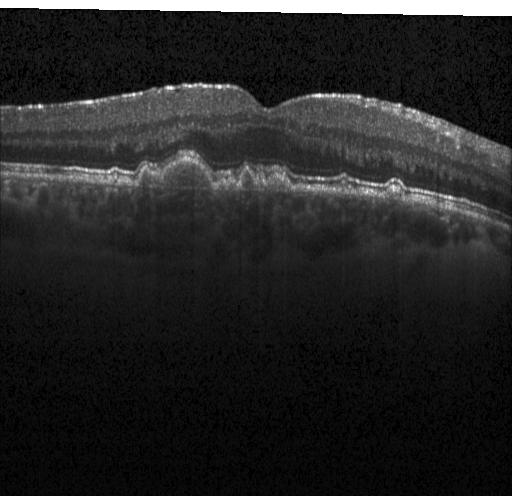 OCT finding: choroidal neovascularization (CNV).